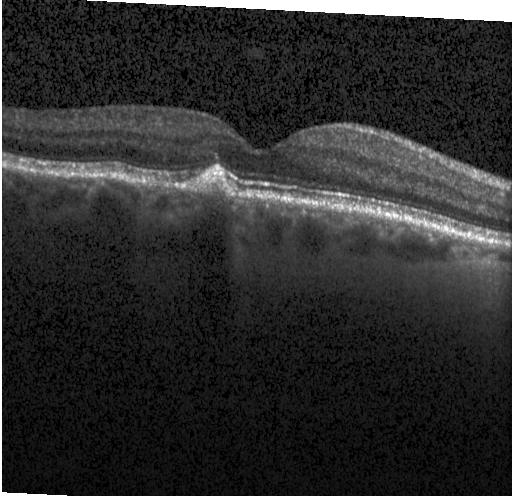 Spectral-domain optical coherence tomography, horizontal scan through the fovea, optical coherence tomography B-scan
Impression: sub-RPE drusenoid deposits.